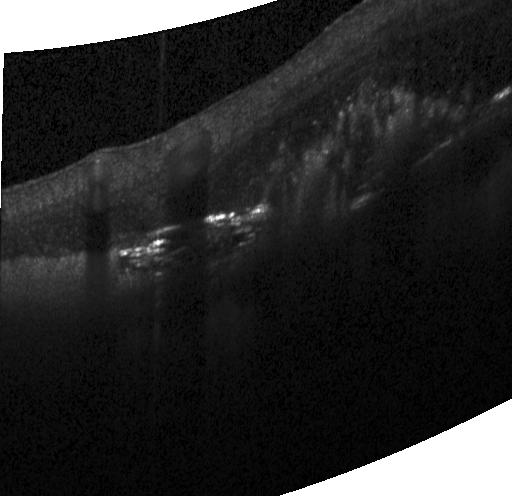 Macular OCT demonstrating a choroidal neovascular membrane.